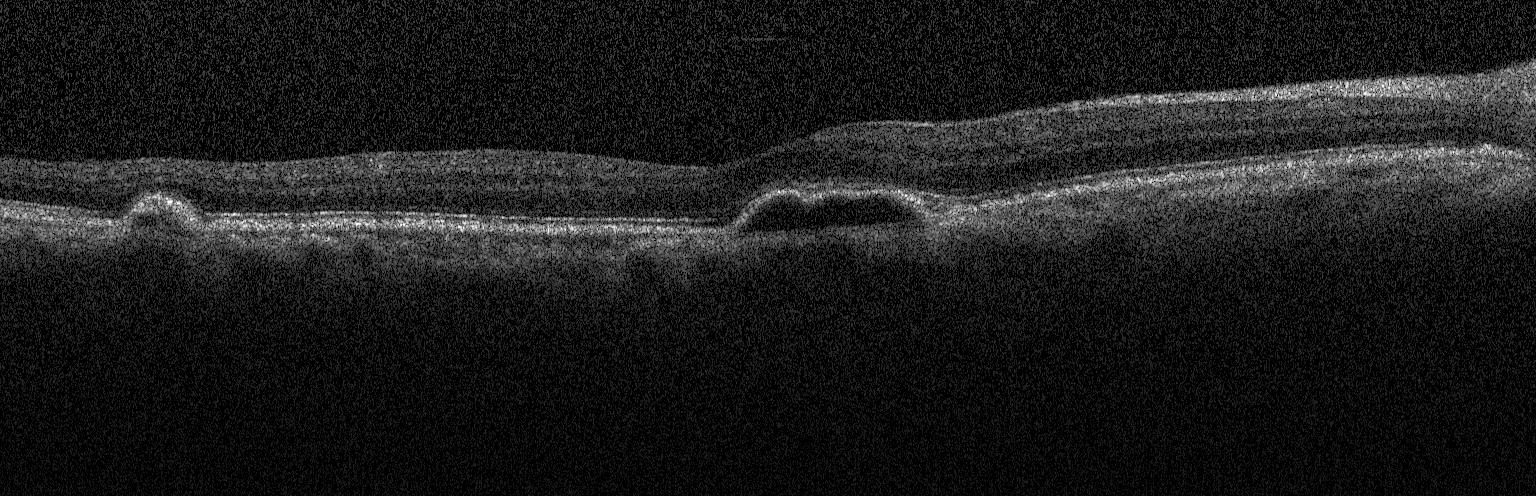
This B-scan demonstrates a choroidal neovascular membrane.